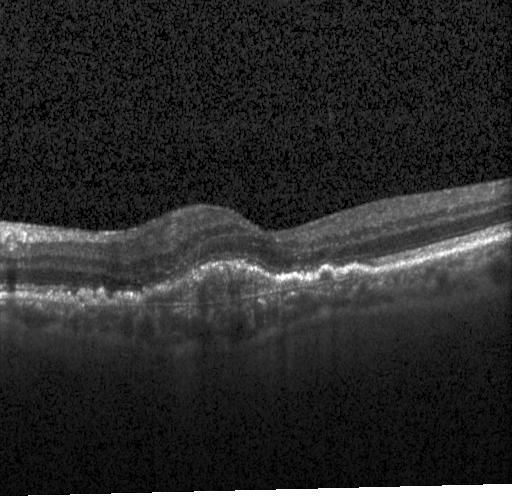

Retinal OCT cross-section · SD-OCT. Macular OCT: choroidal neovascularization.